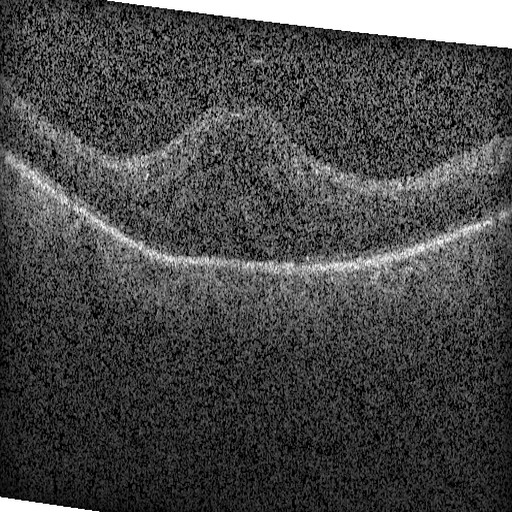
Optical coherence tomography scan, SD-OCT. Assessment: diabetic macular edema.